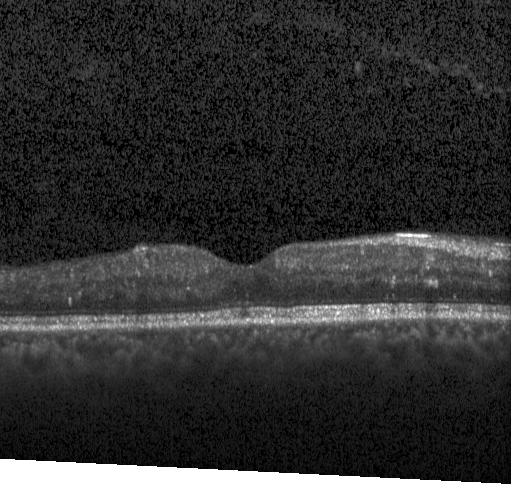
OCT B-scan · instrument: Heidelberg Spectralis. Assessment: diabetic macular edema.